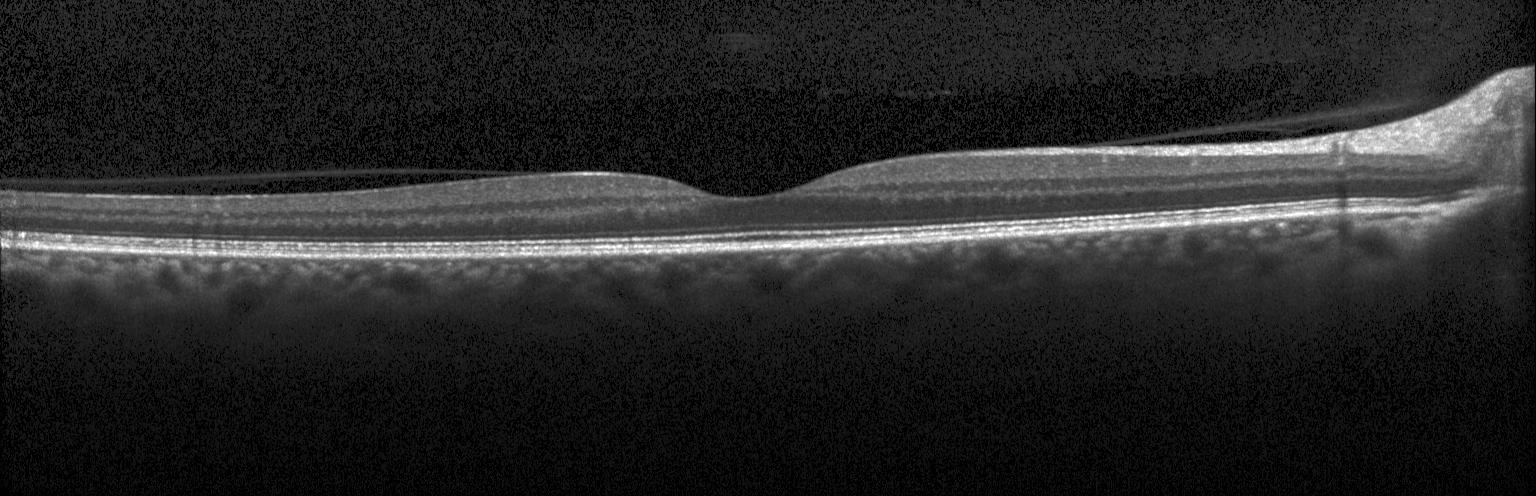
OCT line scan
OCT finding: neither CNV, DME, nor drusen.